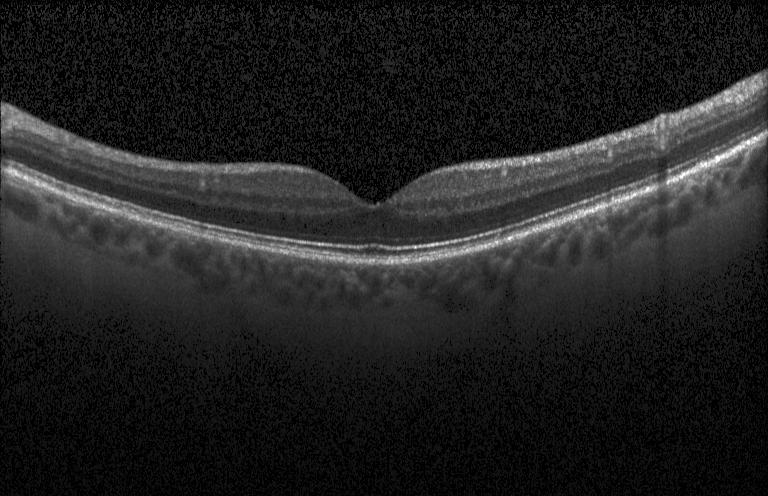

Finding: no evidence of CNV, DME, or drusen.